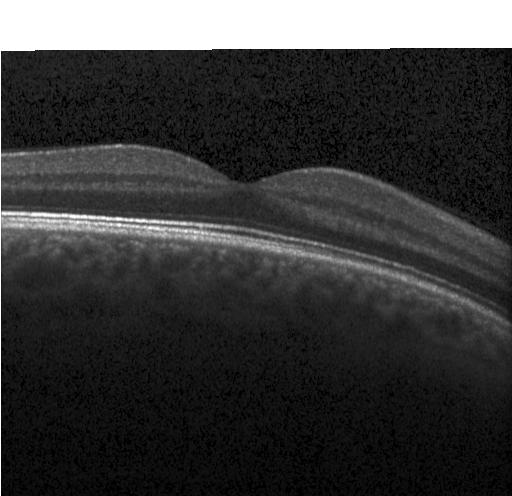

Finding: no CNV, DME, or drusen.